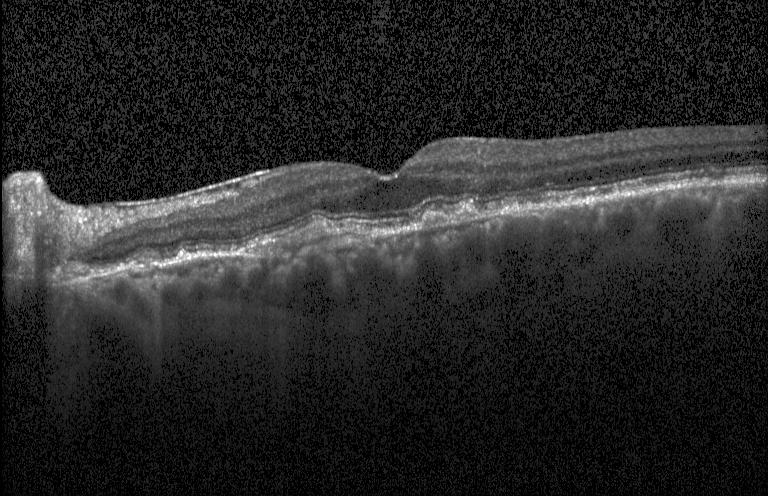

Optical coherence tomography B-scan · Heidelberg Spectralis · SD-OCT — Finding: a choroidal neovascular membrane.